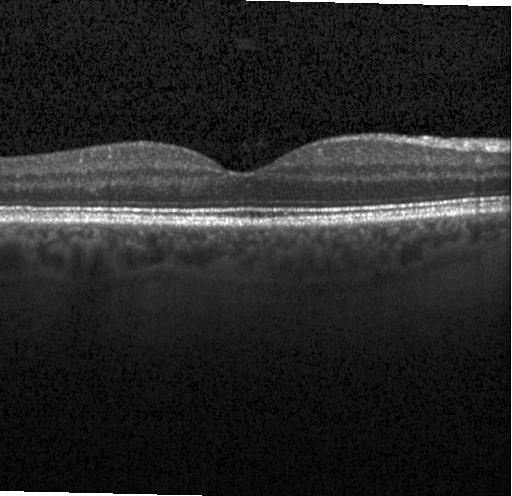 Assessment: no evidence of choroidal neovascularization, diabetic macular edema, or drusen.